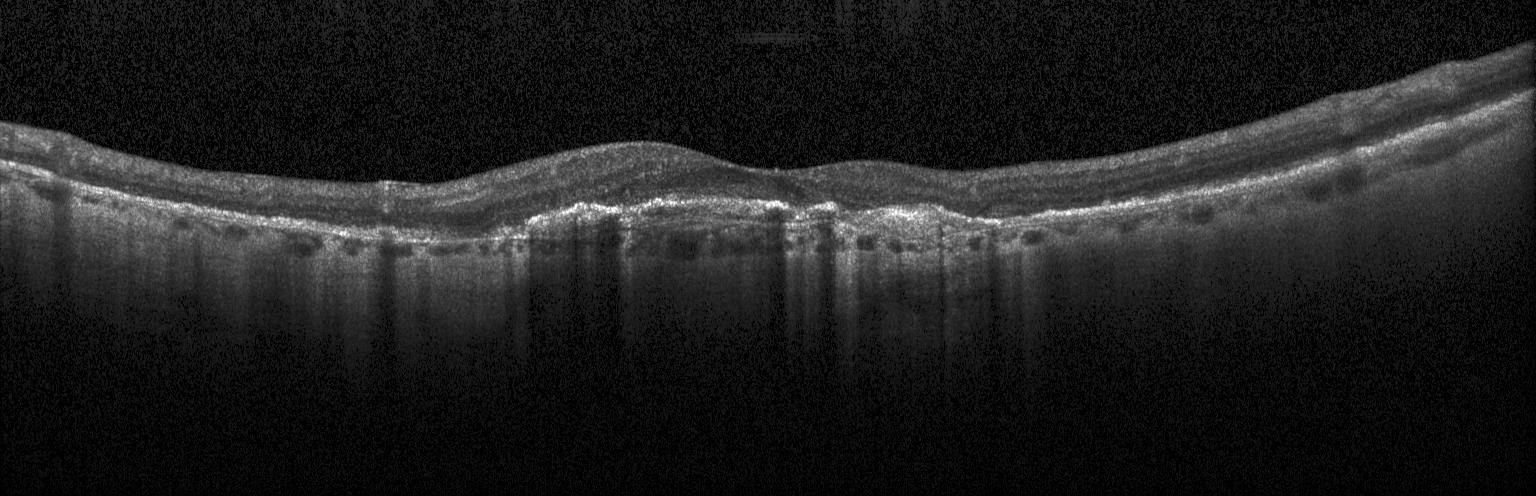

Retinal OCT cross-section.
Finding: CNV.